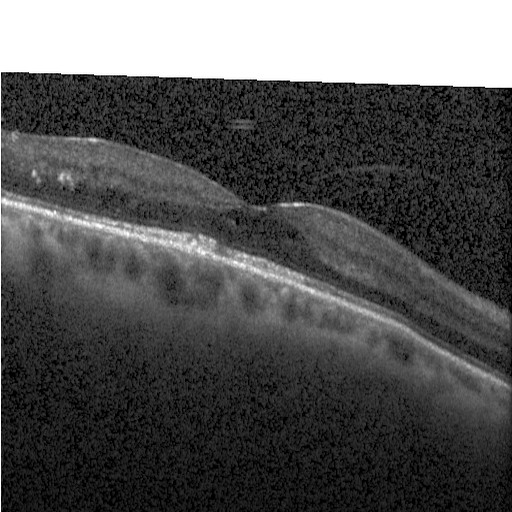 OCT line scan.
Impression: diabetic macular edema.